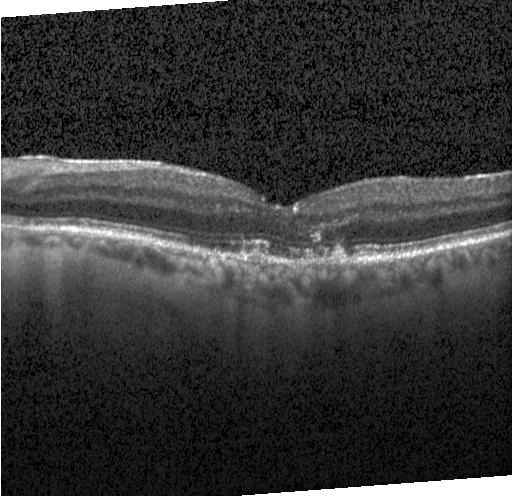 OCT B-scan · spectral-domain optical coherence tomography · centered on the fovea · acquired on a Heidelberg Spectralis.
Macular OCT: choroidal neovascularization.